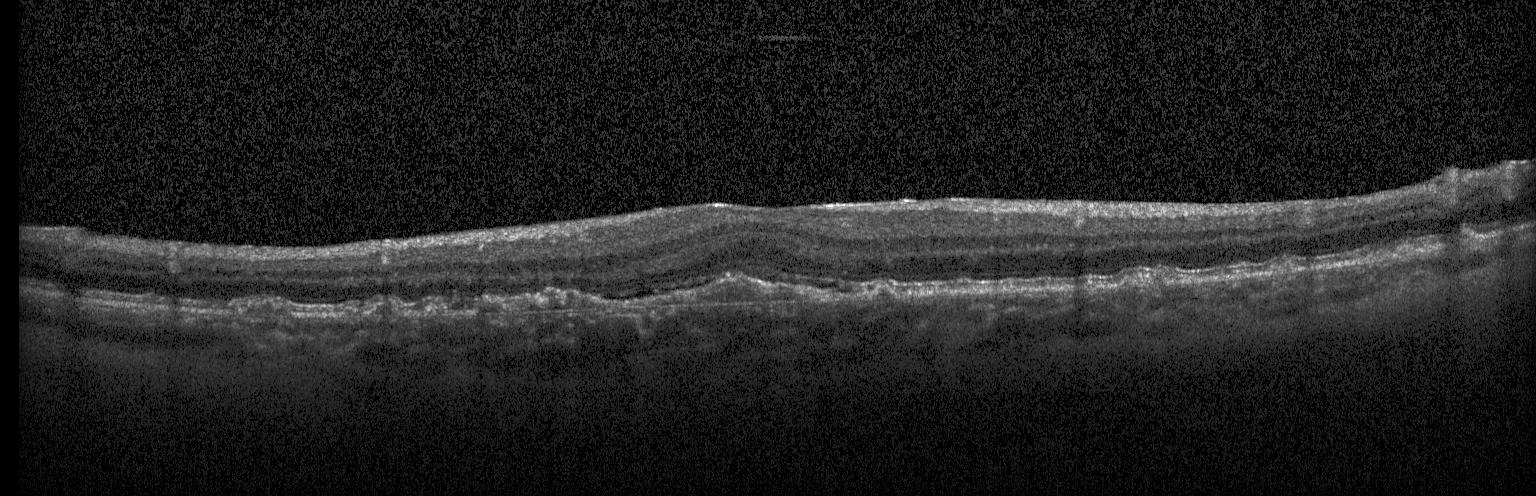 SD-OCT. Optical coherence tomography B-scan.
Assessment: choroidal neovascularization (CNV).